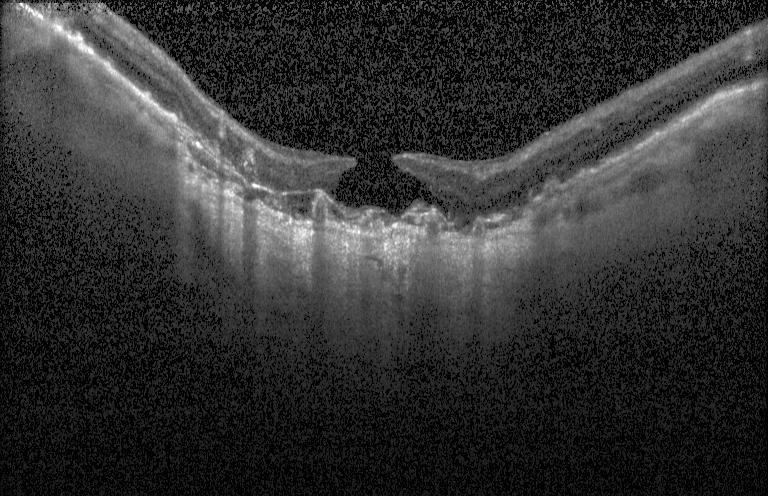 Spectral-domain optical coherence tomography; fovea-centered; retinal OCT B-scan; Heidelberg Spectralis.
This B-scan demonstrates a choroidal neovascular membrane.